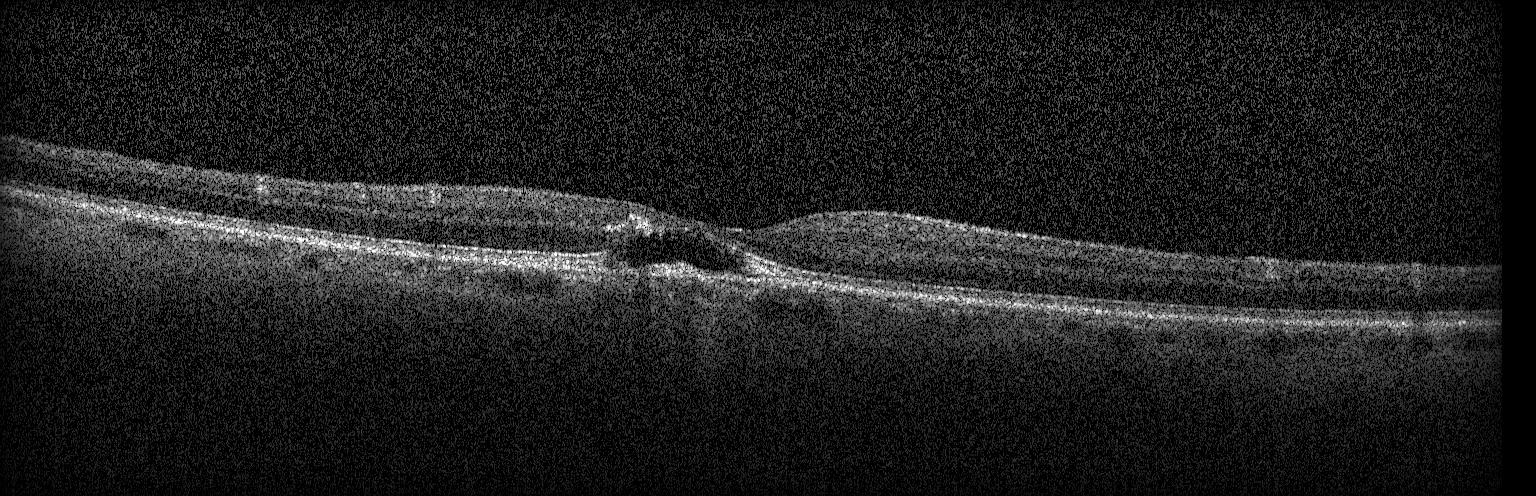
Retinal OCT B-scan.
Impression: a choroidal neovascular membrane.